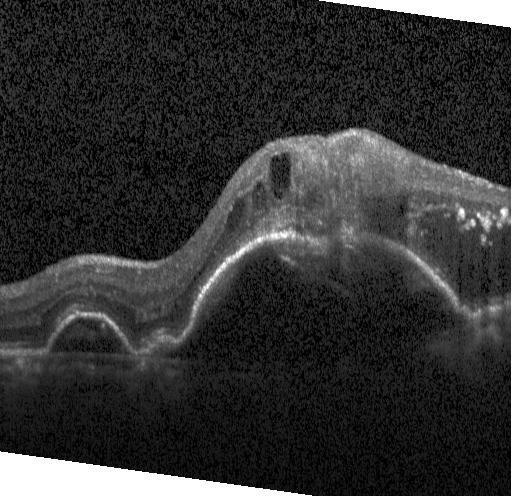

Diagnosis: a choroidal neovascular membrane.